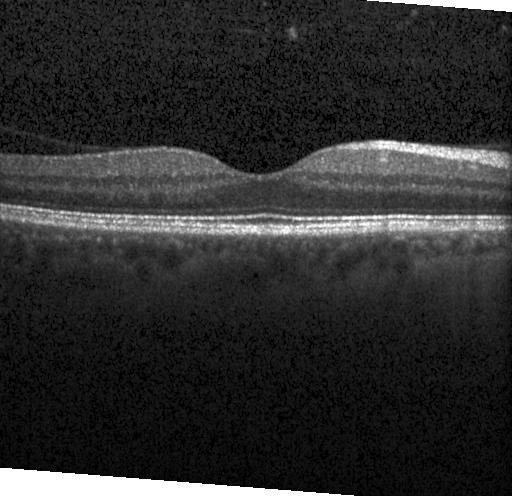

Optical coherence tomography B-scan · through the macula · spectral-domain optical coherence tomography.
Finding: no evidence of CNV, DME, or drusen.